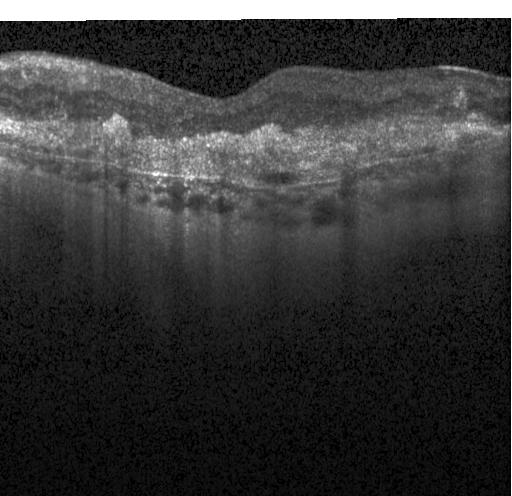 Finding: choroidal neovascularization (CNV).